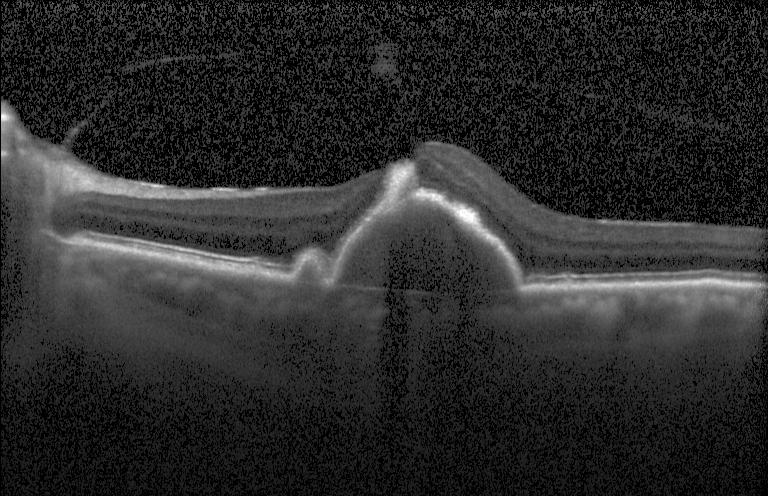 Optical coherence tomography B-scan.
Macular OCT: choroidal neovascularization.